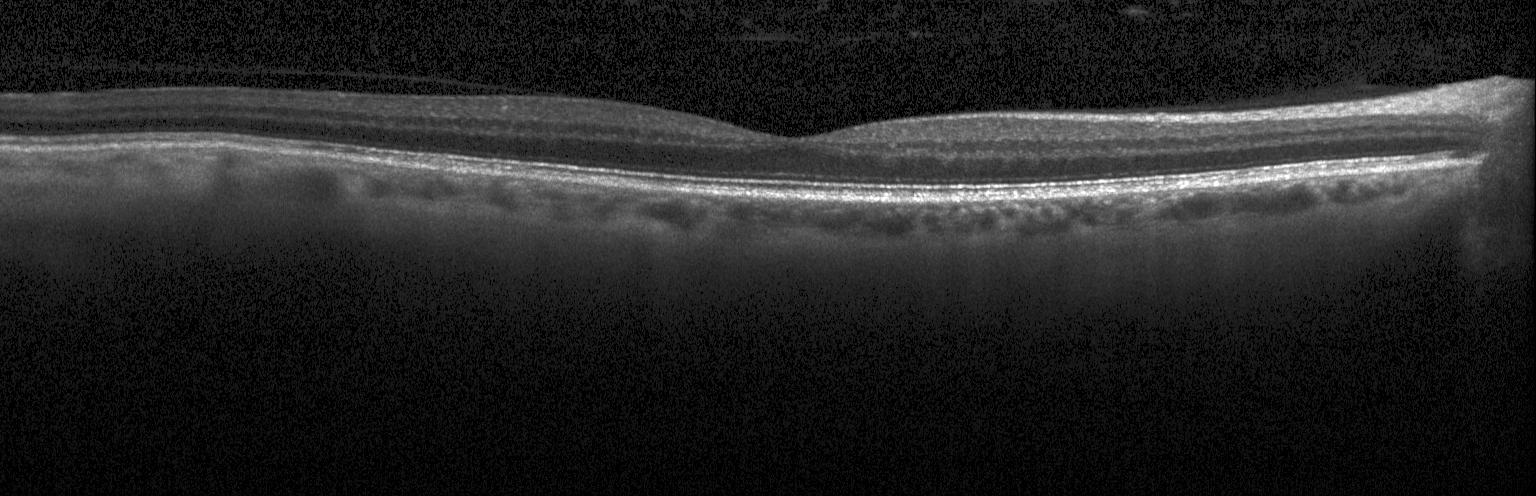

Retinal OCT cross-section.
Finding: no choroidal neovascularization, no diabetic macular edema, and no drusen.